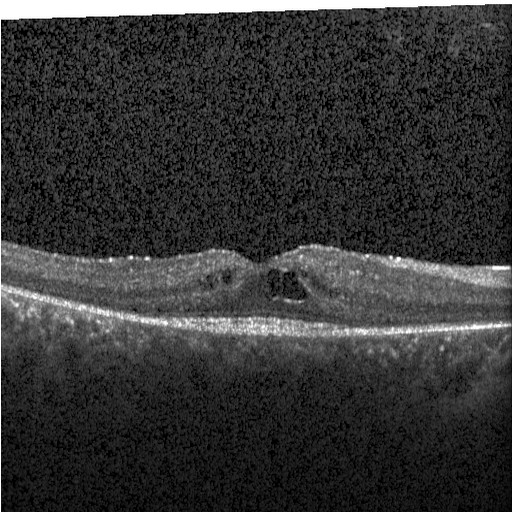

OCT line scan, instrument: Heidelberg Spectralis, spectral-domain optical coherence tomography — Dx: DME.